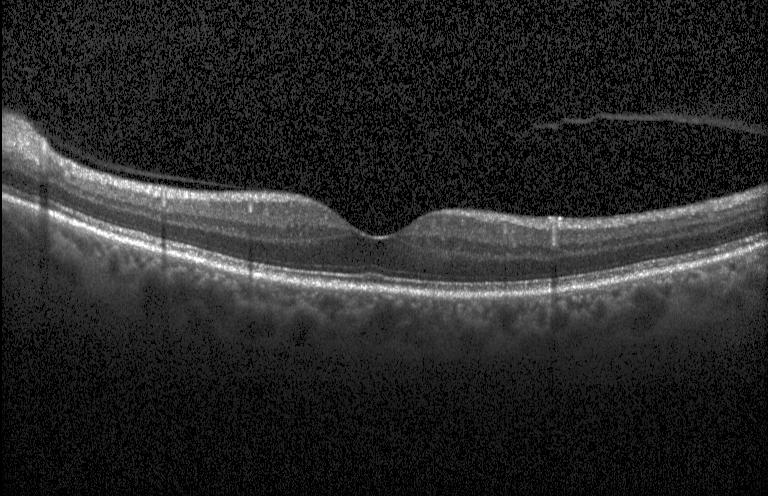
Acquired on a Heidelberg Spectralis, macular scan, spectral-domain OCT, retinal OCT B-scan.
Impression: no CNV, DME, or drusen.